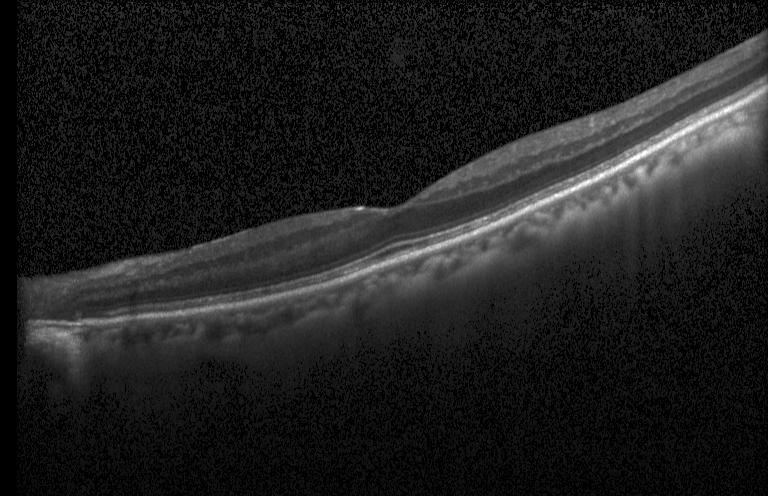

Optical coherence tomography scan — The scan shows no evidence of choroidal neovascularization, diabetic macular edema, or drusen.